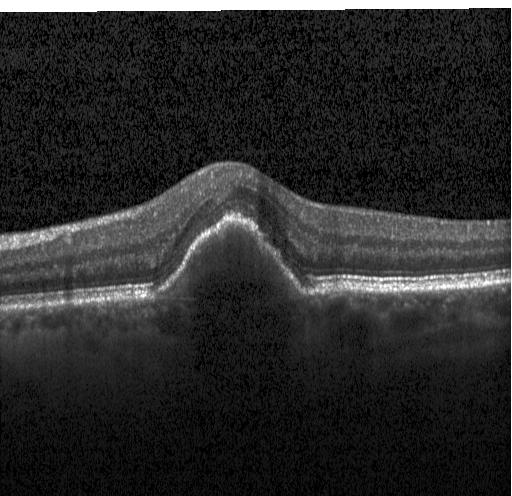 Spectral-domain OCT B-scan: CNV.